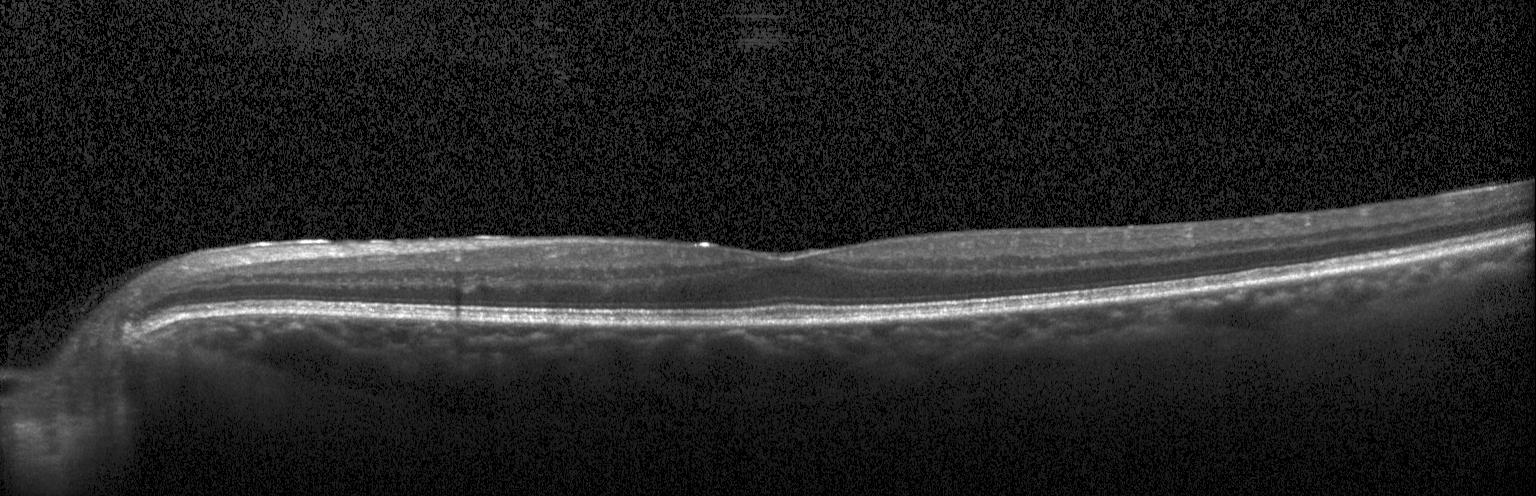

OCT scan showing no CNV, no DME, and no drusen.